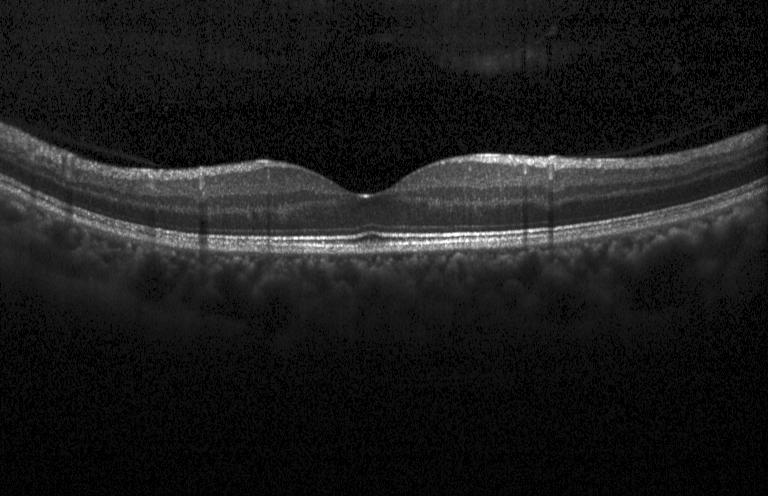

Diagnosis: no CNV, no DME, and no drusen.